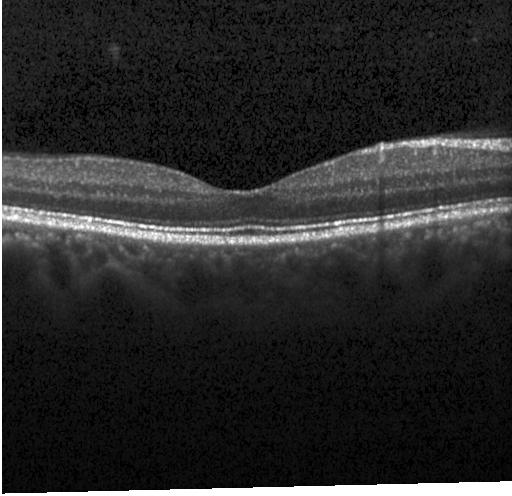

Optical coherence tomography B-scan — No choroidal neovascularization, diabetic macular edema, or drusen.